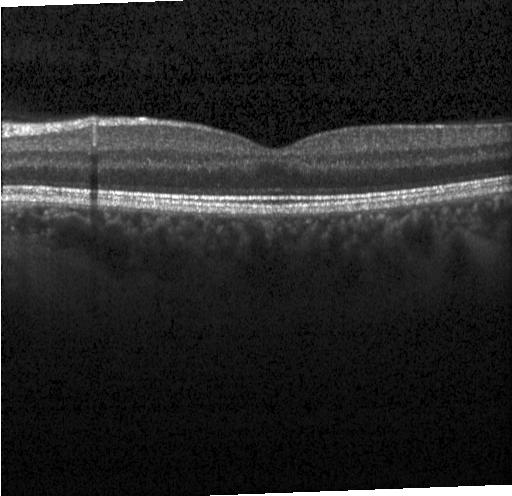 Optical coherence tomography B-scan
Diagnosis: neither choroidal neovascularization, diabetic macular edema, nor drusen.